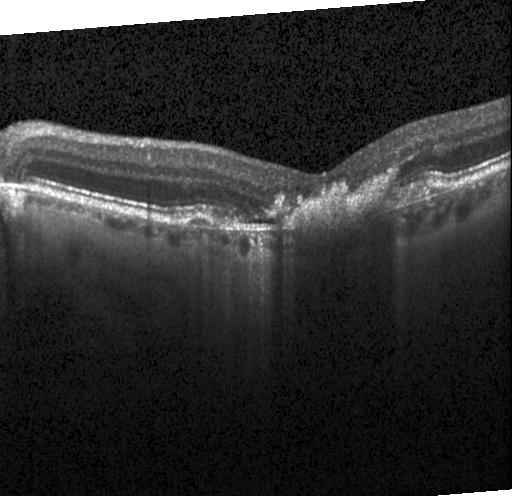
OCT B-scan
This B-scan demonstrates a choroidal neovascular membrane.